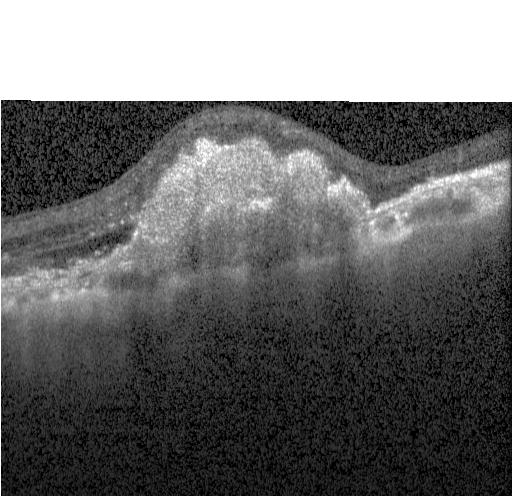
Heidelberg Spectralis OCT system · optical coherence tomography scan
This B-scan demonstrates choroidal neovascularization.